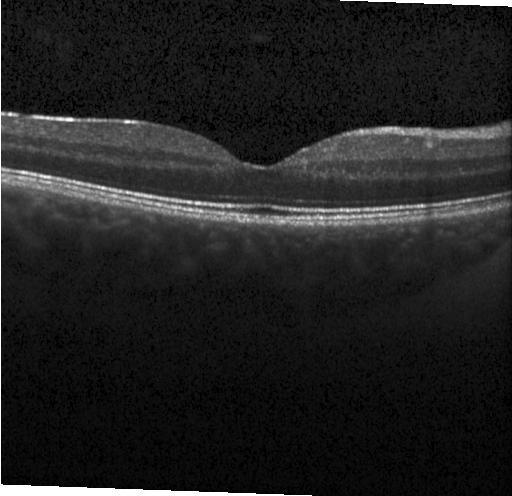
Spectral-domain optical coherence tomography · acquired on a Heidelberg Spectralis · fovea-centered · optical coherence tomography scan.
Impression: no choroidal neovascularization, diabetic macular edema, or drusen.